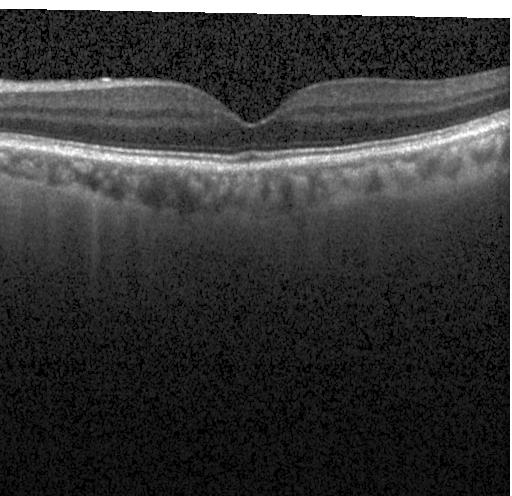 OCT line scan. The scan shows neither CNV, DME, nor drusen.